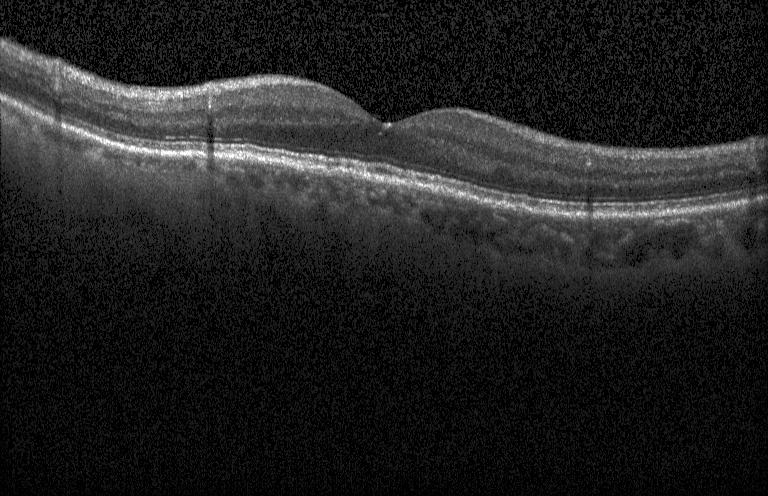

Diagnosis: no choroidal neovascularization, diabetic macular edema, or drusen.